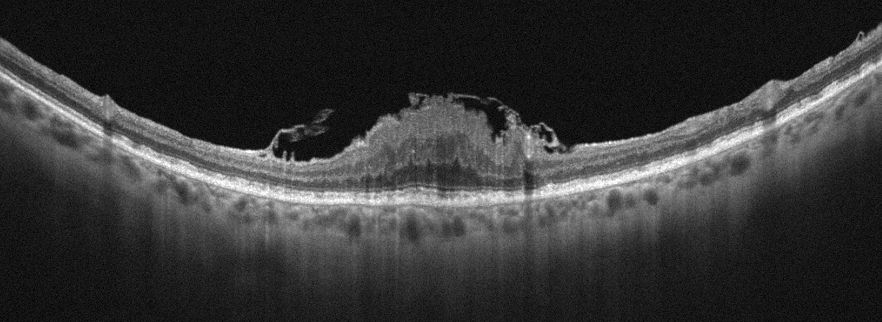 Optical coherence tomography B-scan; macular scan; instrument: Optovue Avanti RTVue XR. Impression: ERM.